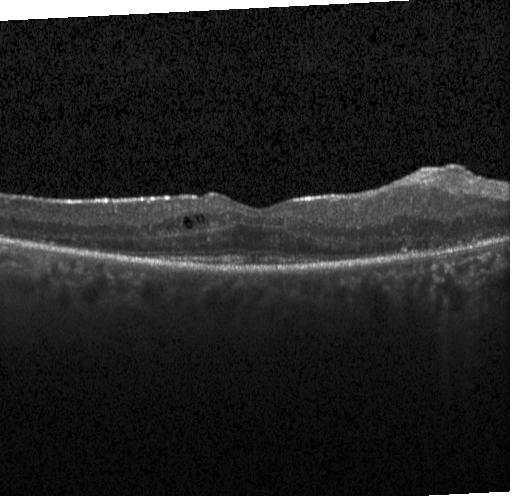

Optical coherence tomography B-scan, through the macula.
Macular OCT: diabetic macular edema (DME).